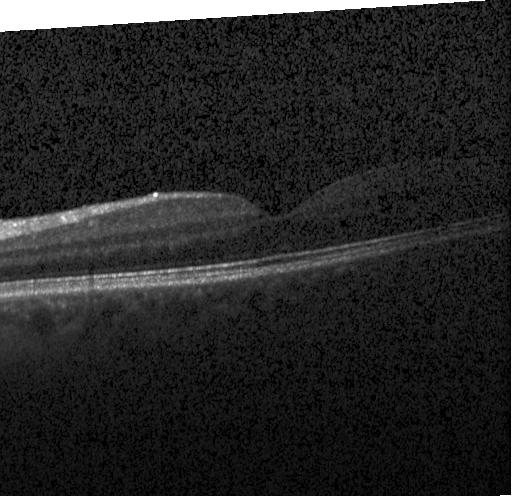 Spectral-domain OCT. Horizontal scan through the fovea. Instrument: Heidelberg Spectralis. Optical coherence tomography B-scan
Impression: no evidence of choroidal neovascularization, diabetic macular edema, or drusen.